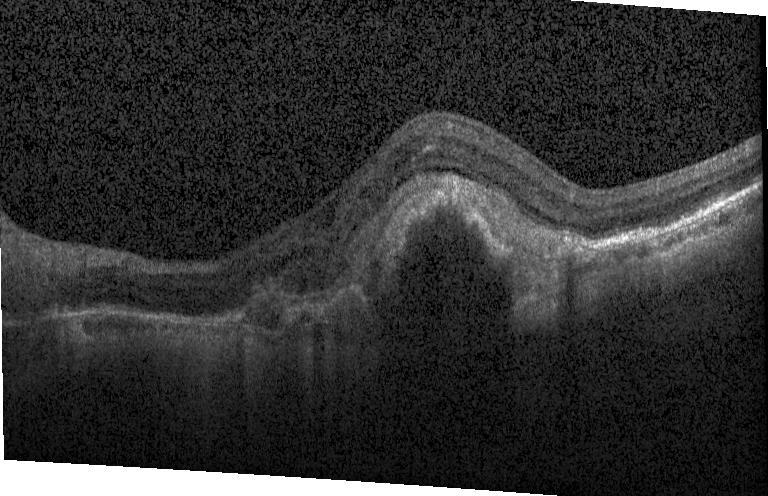

Optical coherence tomography scan, Heidelberg Spectralis, spectral-domain optical coherence tomography, through the macula — Choroidal neovascularization.